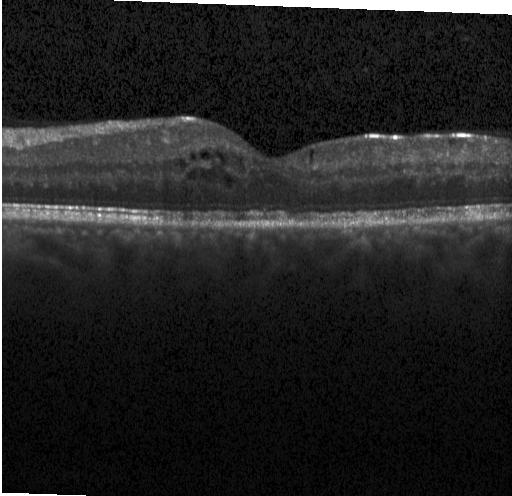 Optical coherence tomography scan. The scan shows diabetic macular edema.